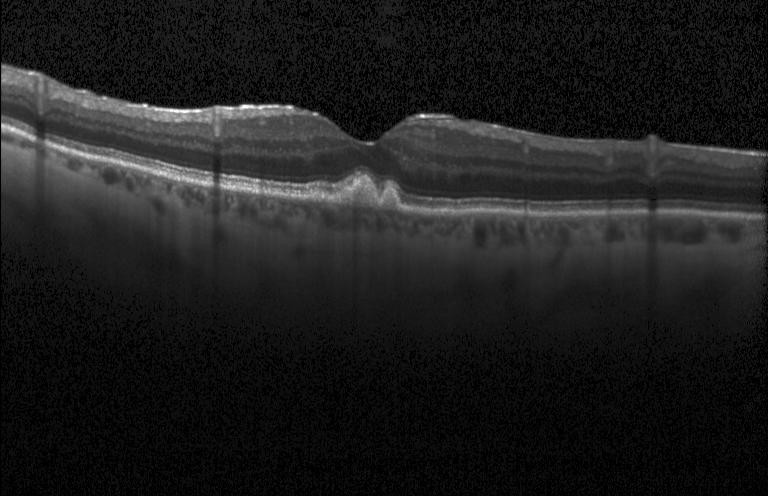 Macular OCT: multiple drusen.